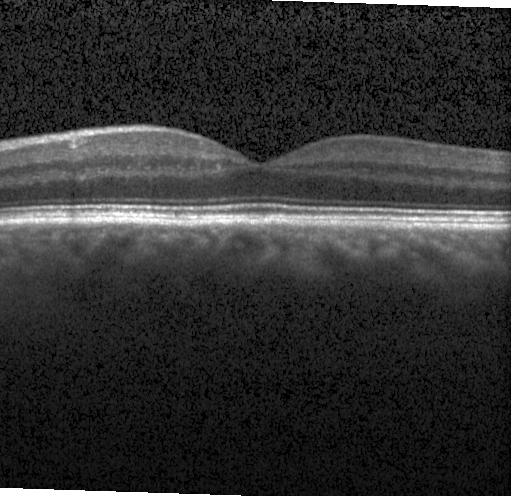 Retinal OCT cross-section showing neither choroidal neovascularization, diabetic macular edema, nor drusen.